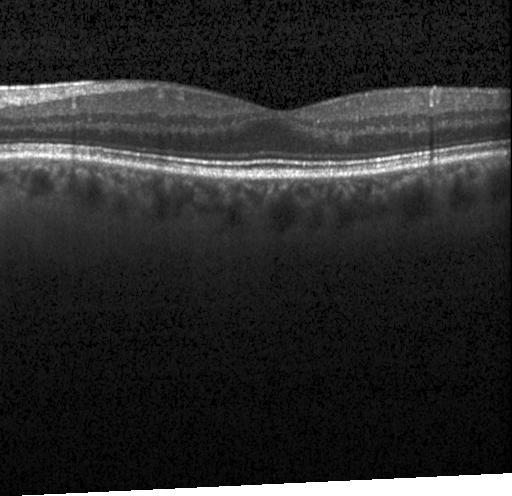

Macular OCT demonstrating no choroidal neovascularization, no diabetic macular edema, and no drusen.